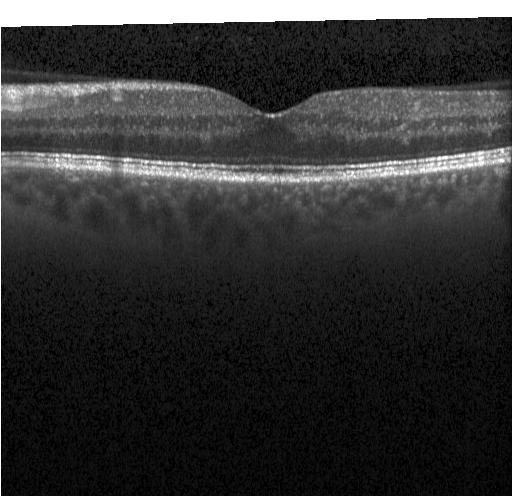
SD-OCT. Optical coherence tomography B-scan. Heidelberg Spectralis OCT system. Horizontal scan through the fovea.
OCT finding: no choroidal neovascularization, diabetic macular edema, or drusen.